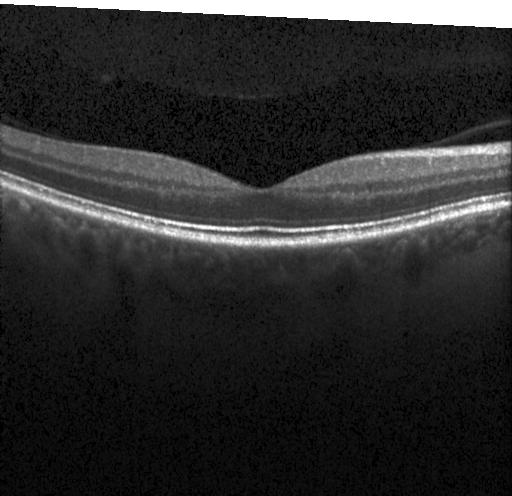 OCT line scan. Heidelberg Spectralis — Macular OCT: no choroidal neovascularization, no diabetic macular edema, and no drusen.